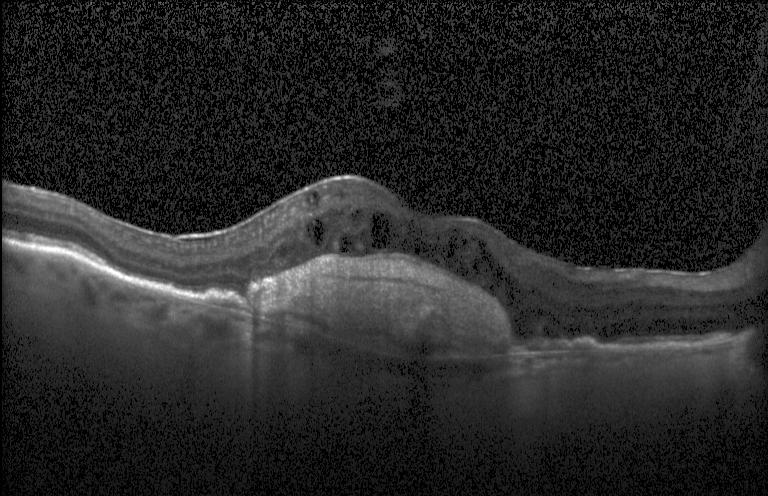
OCT line scan · acquired on a Heidelberg Spectralis · centered on the fovea · SD-OCT.
Assessment: a choroidal neovascular membrane.